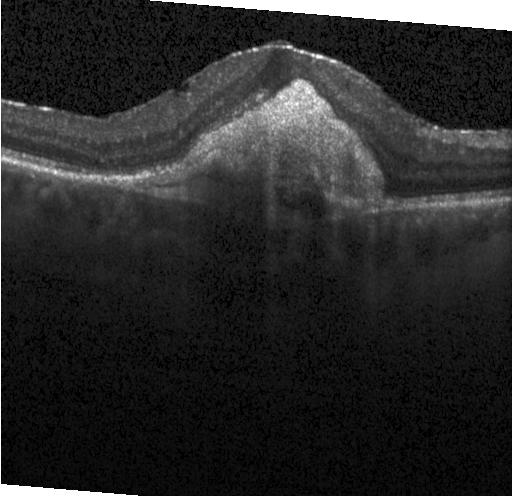 Retinal OCT B-scan, Heidelberg Spectralis — Finding: a choroidal neovascular membrane.